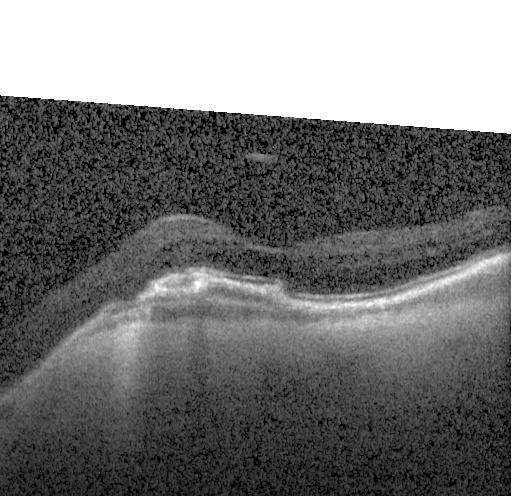
Dx: choroidal neovascularization.